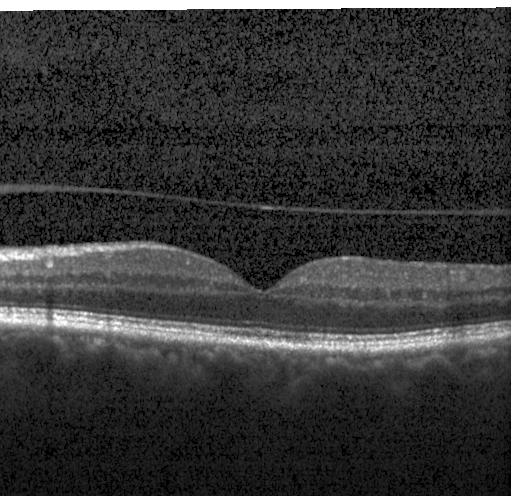
OCT B-scan. SD-OCT — Dx: no choroidal neovascularization, no diabetic macular edema, and no drusen.